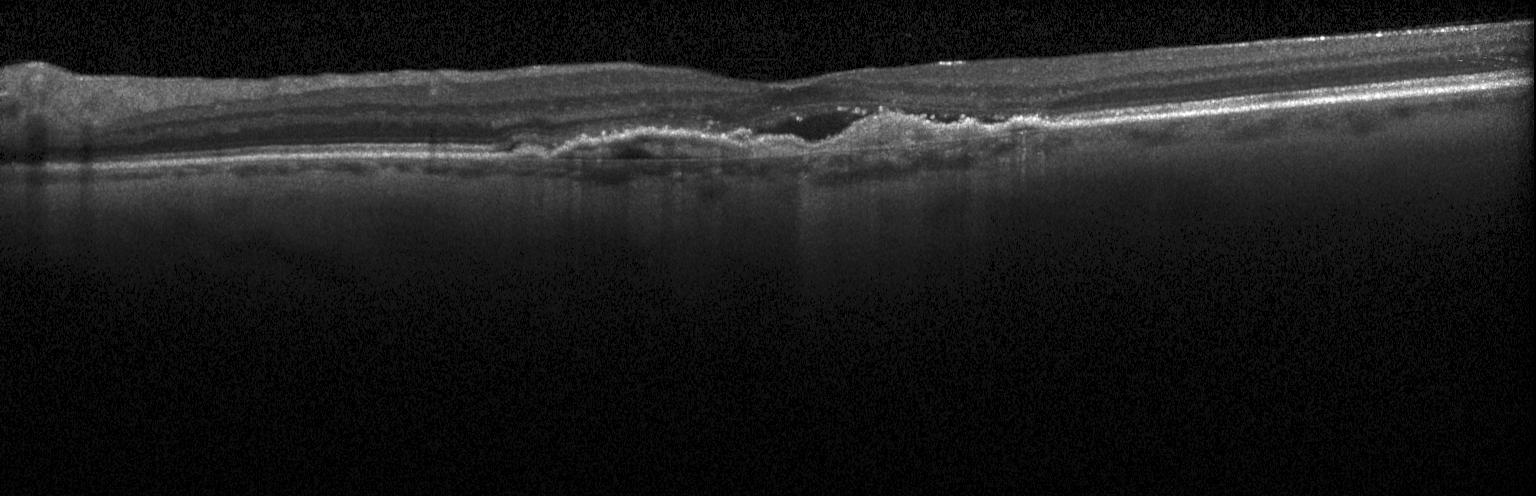 Finding: CNV.